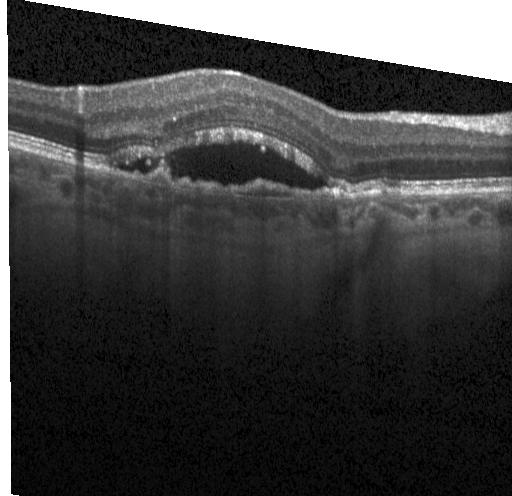 Diagnosis: choroidal neovascularization (CNV).